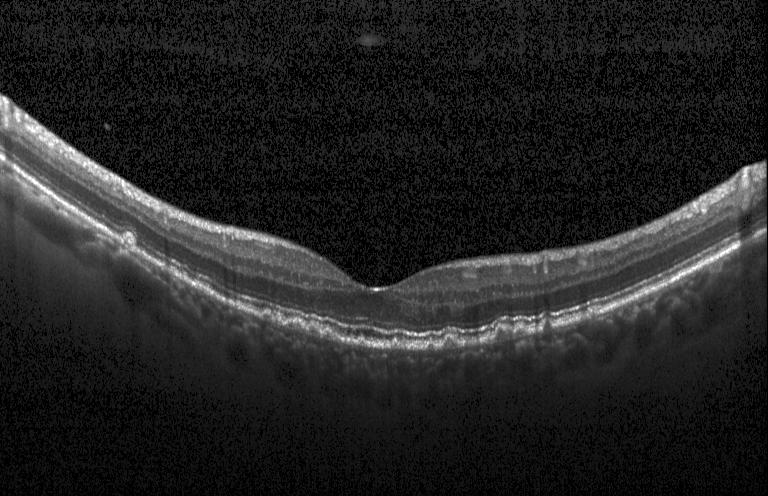
Heidelberg Spectralis OCT system; optical coherence tomography scan; centered on the fovea.
Impression: multiple drusen.